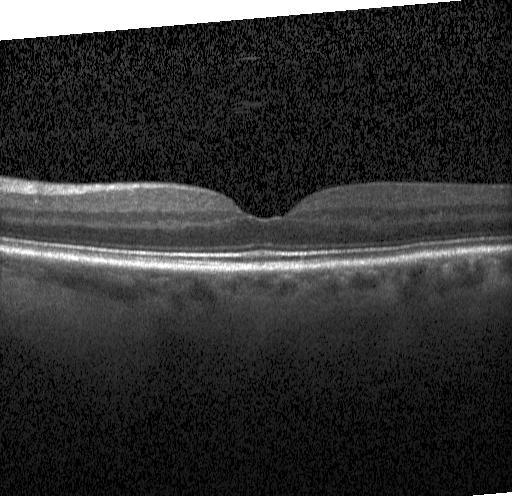

This B-scan demonstrates no evidence of choroidal neovascularization, diabetic macular edema, or drusen.